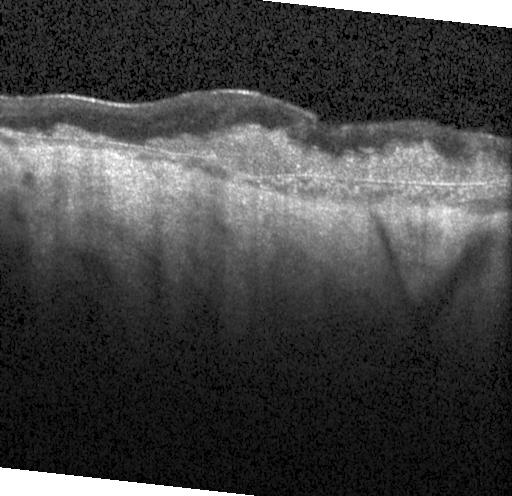 Diagnosis: a choroidal neovascular membrane.